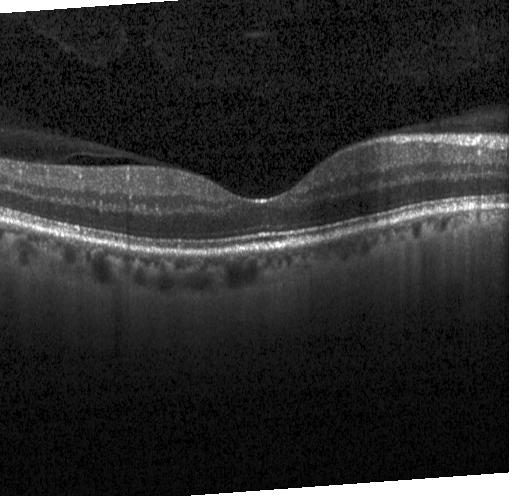

Retinal OCT cross-section showing no choroidal neovascularization, diabetic macular edema, or drusen.